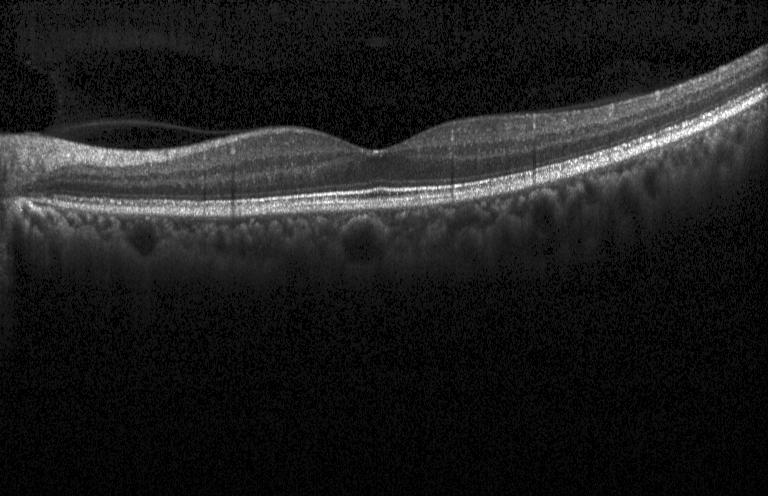

Macular OCT: no choroidal neovascularization, diabetic macular edema, or drusen.